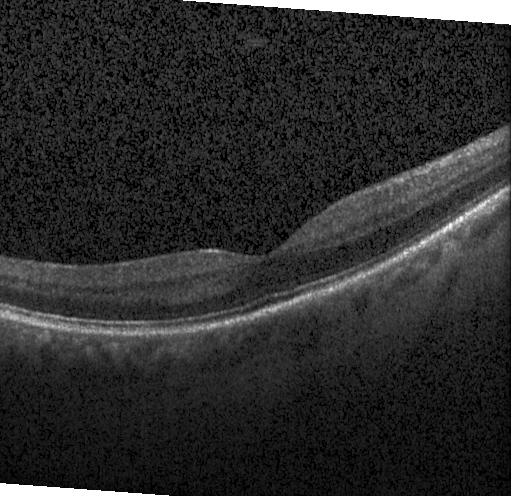
Dx: no evidence of choroidal neovascularization, diabetic macular edema, or drusen.